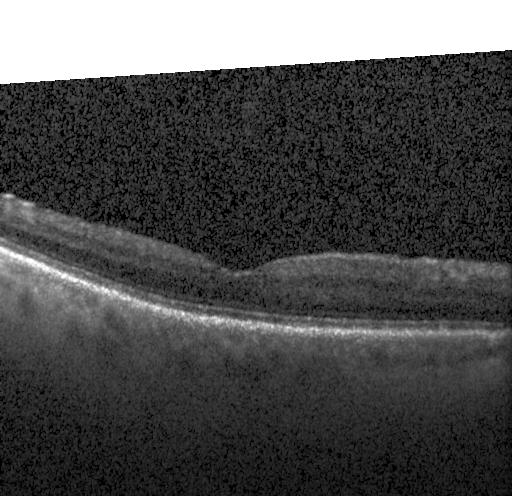

Impression: no choroidal neovascularization, no diabetic macular edema, and no drusen.